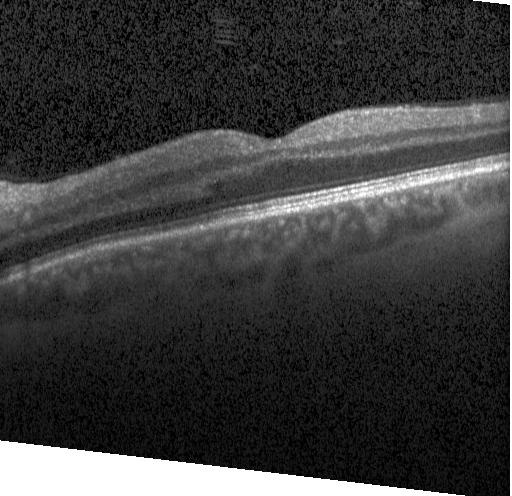
Retinal OCT cross-section, spectral-domain optical coherence tomography
Diagnosis: no evidence of CNV, DME, or drusen.